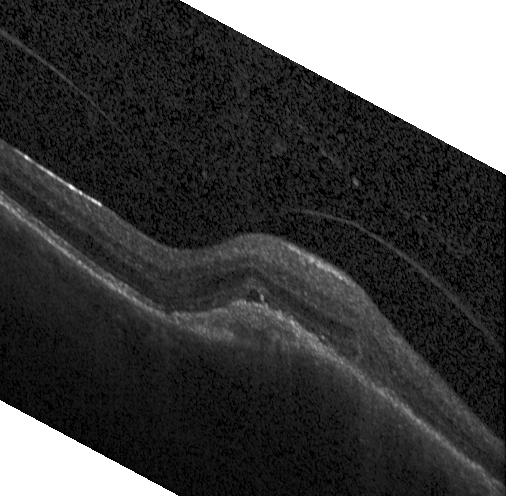

Macular OCT demonstrating choroidal neovascularization (CNV).